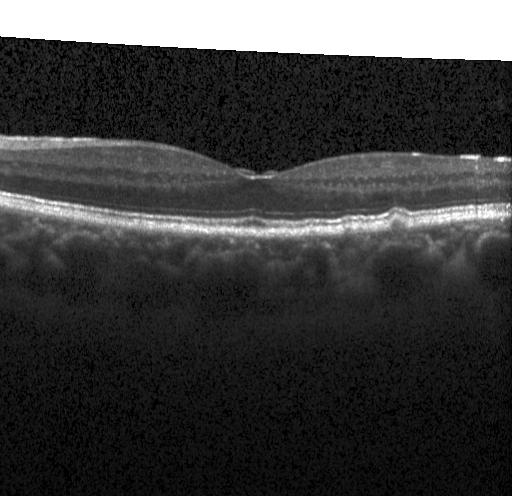
Diagnosis: sub-RPE drusenoid deposits.